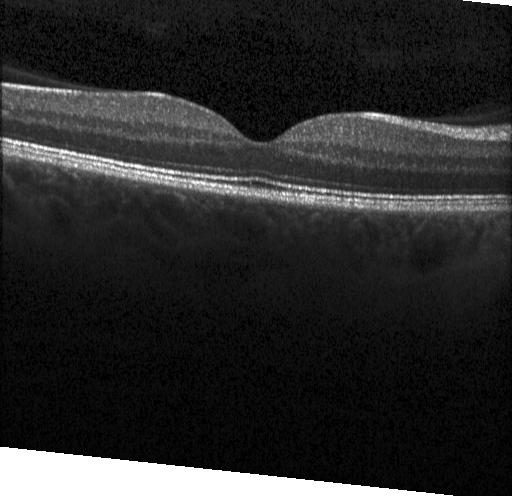

OCT line scan; horizontal scan through the fovea — This B-scan demonstrates no CNV, no DME, and no drusen.